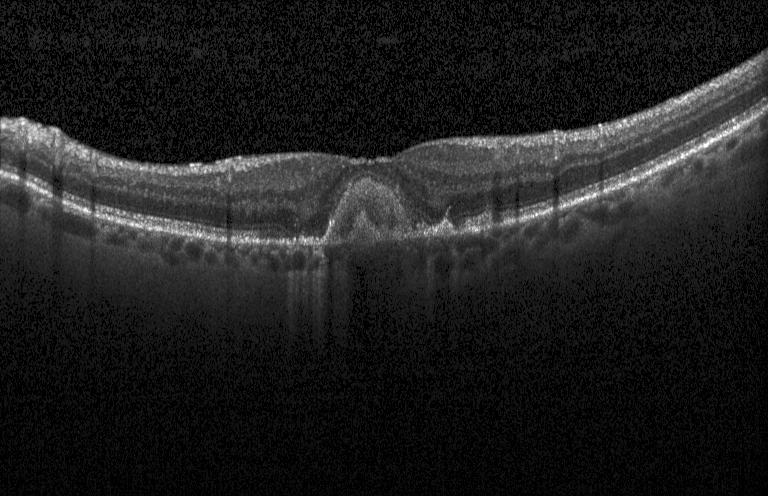
Dx: a choroidal neovascular membrane.